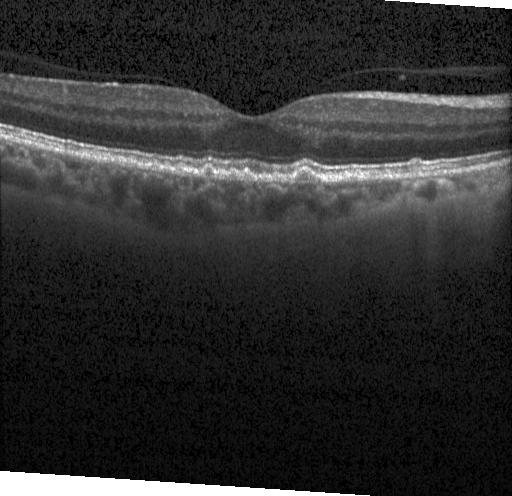

OCT B-scan — OCT finding: sub-RPE drusenoid deposits.